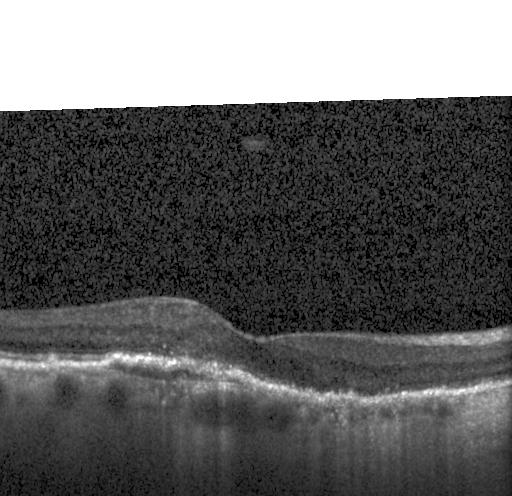 Retinal OCT cross-section — Impression: a choroidal neovascular membrane.